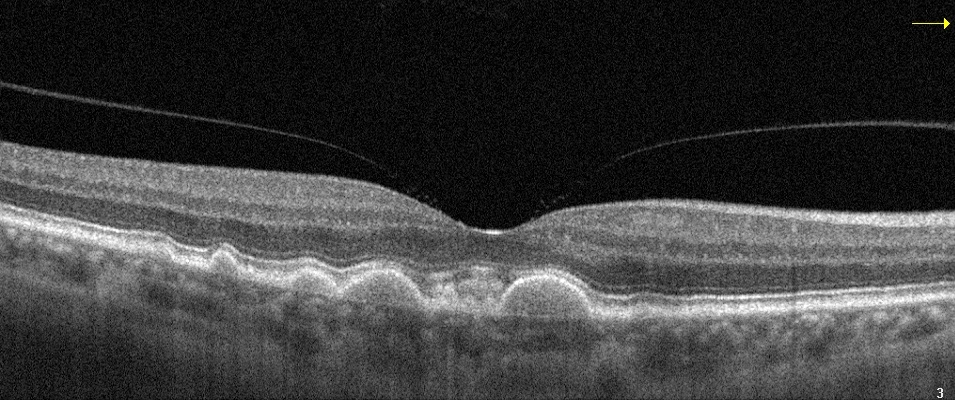 Age-related macular degeneration (AMD).